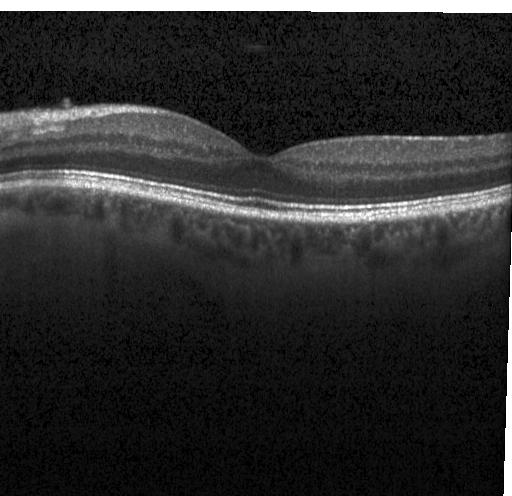 Spectral-domain OCT · OCT B-scan · horizontal scan through the fovea.
This B-scan demonstrates no evidence of choroidal neovascularization, diabetic macular edema, or drusen.